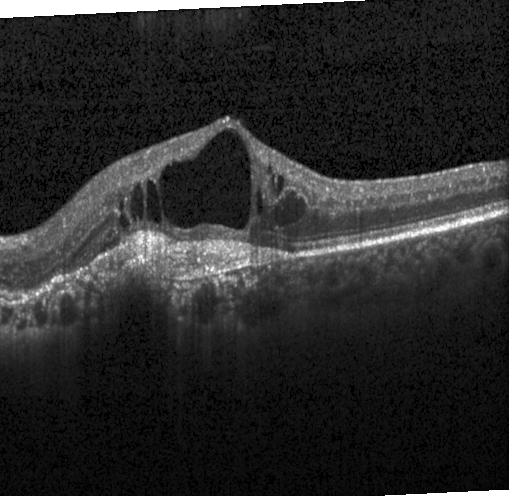 Spectral-domain OCT B-scan: a choroidal neovascular membrane.